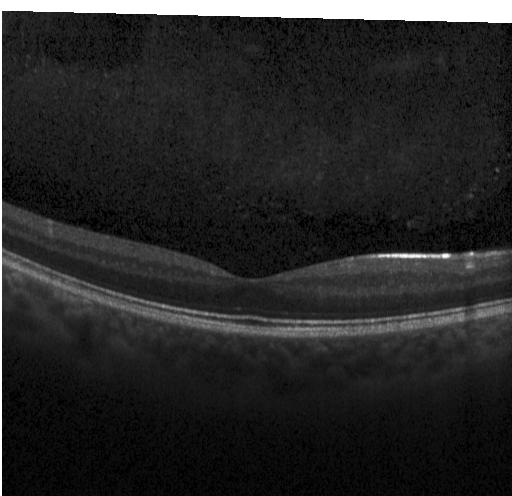 Finding: no evidence of CNV, DME, or drusen.